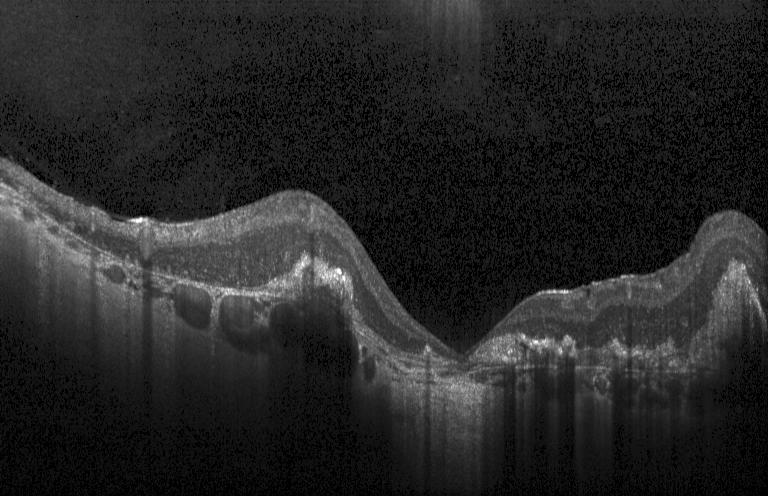 This B-scan demonstrates choroidal neovascularization (CNV).